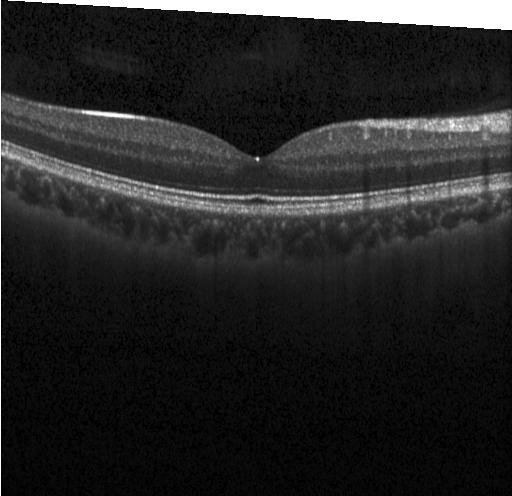

OCT finding: neither choroidal neovascularization, diabetic macular edema, nor drusen.